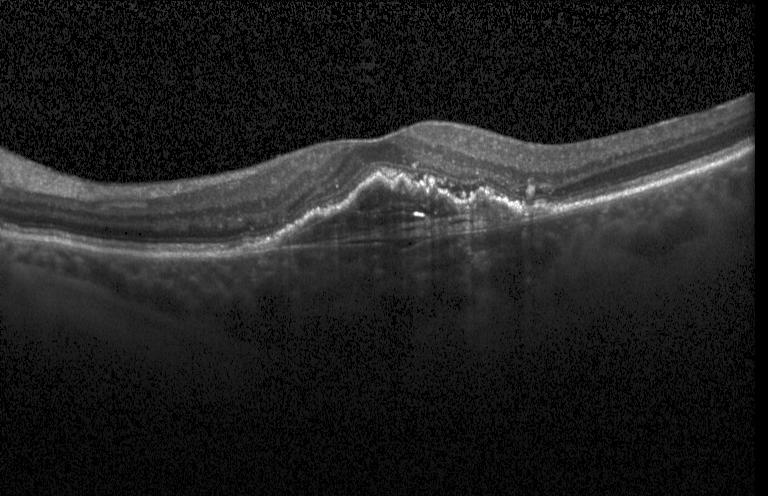 Diagnosis: choroidal neovascularization.